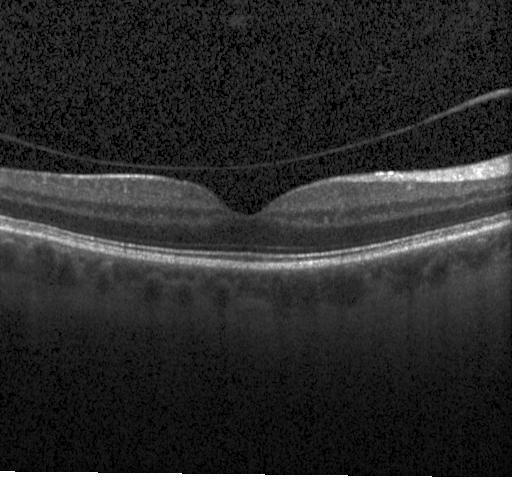

Macular scan · retinal OCT cross-section · acquired on a Heidelberg Spectralis · spectral-domain optical coherence tomography. OCT finding: no choroidal neovascularization, no diabetic macular edema, and no drusen.